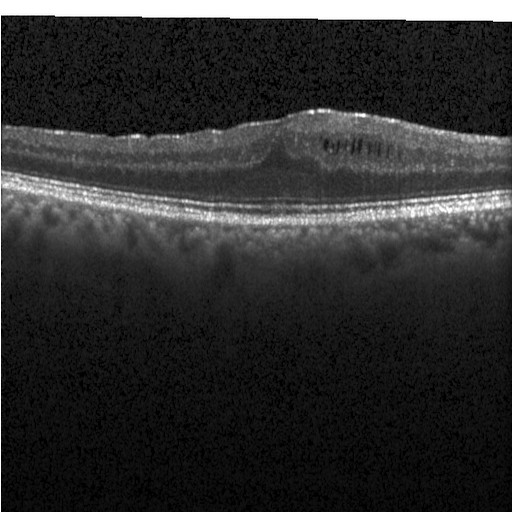
Finding: DME.